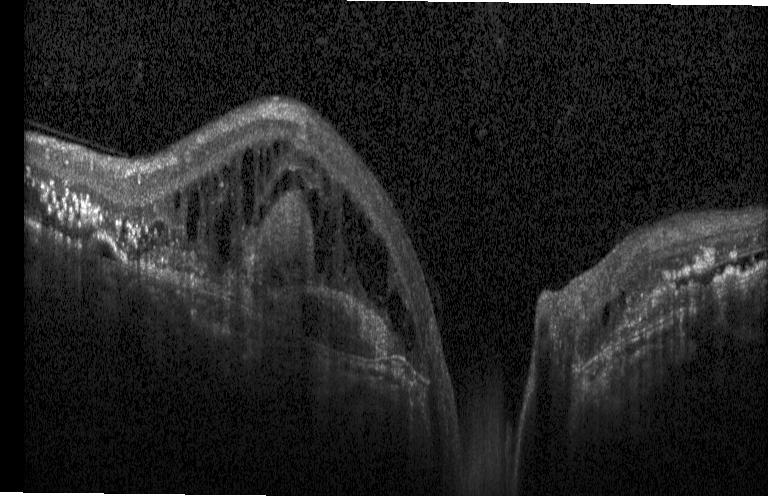
Finding: choroidal neovascularization.